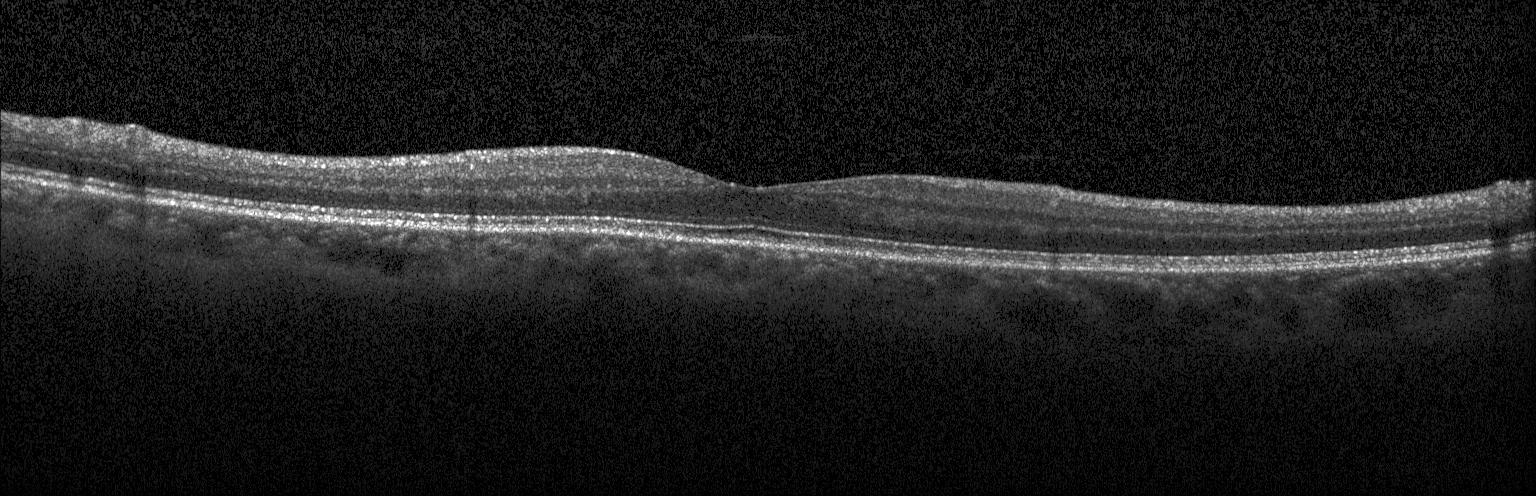

Assessment: neither CNV, DME, nor drusen.